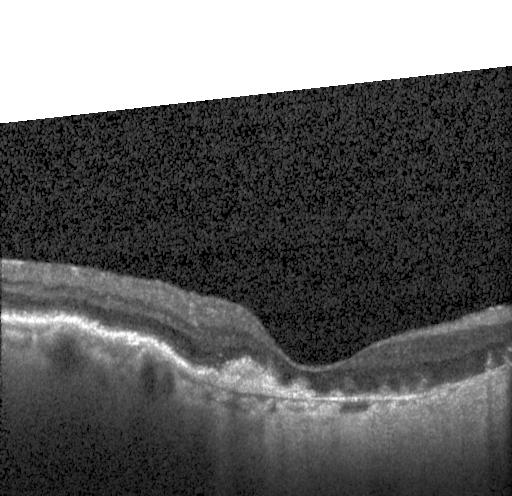
Spectral-domain OCT, retinal OCT B-scan, fovea-centered — Macular OCT: choroidal neovascularization (CNV).